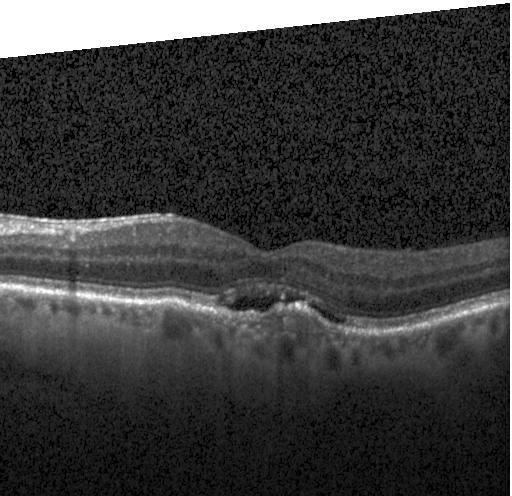
Retinal OCT B-scan
A choroidal neovascular membrane.